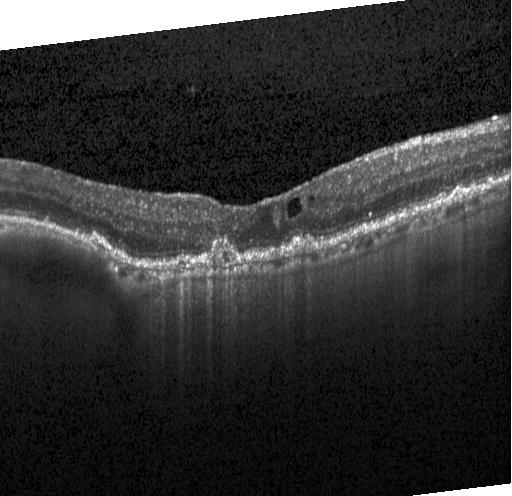

Finding: CNV.